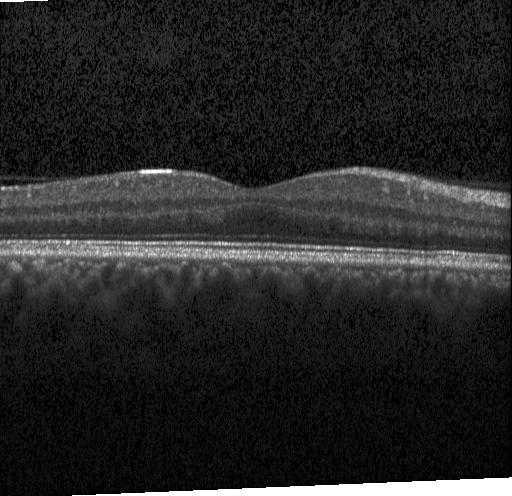 Impression: neither CNV, DME, nor drusen.